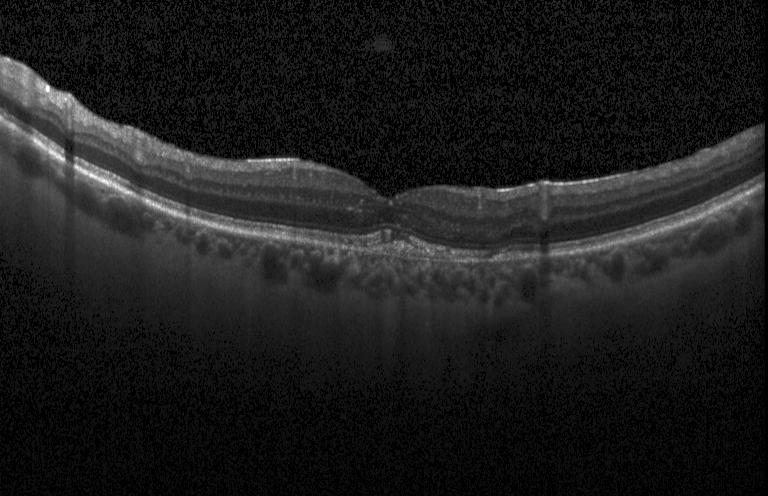
Impression: a choroidal neovascular membrane.